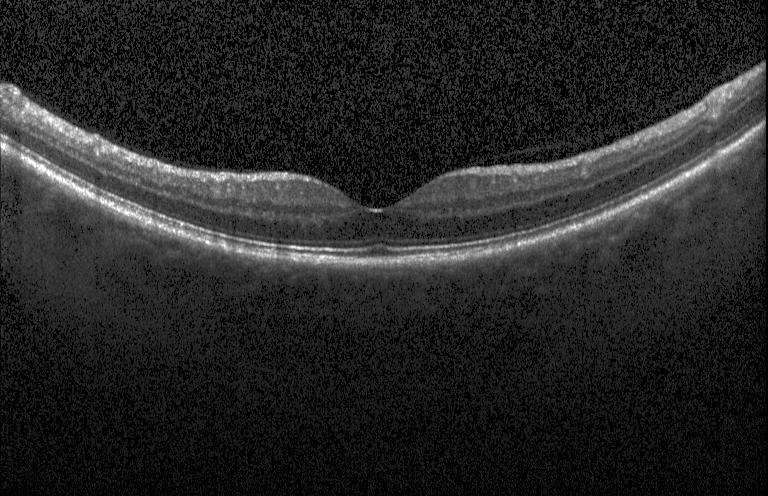
Retinal OCT cross-section; fovea-centered; spectral-domain OCT.
Assessment: no evidence of choroidal neovascularization, diabetic macular edema, or drusen.